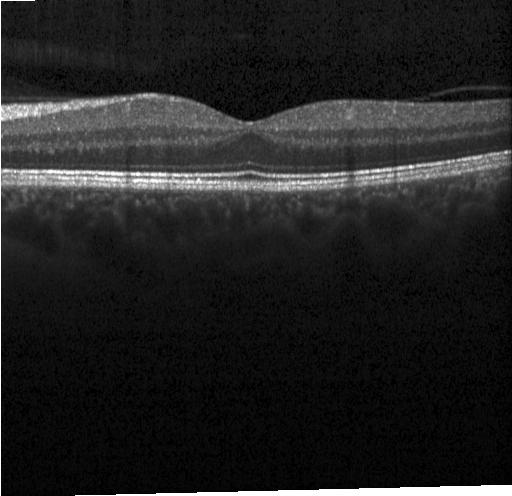
Retinal OCT cross-section.
Finding: neither CNV, DME, nor drusen.